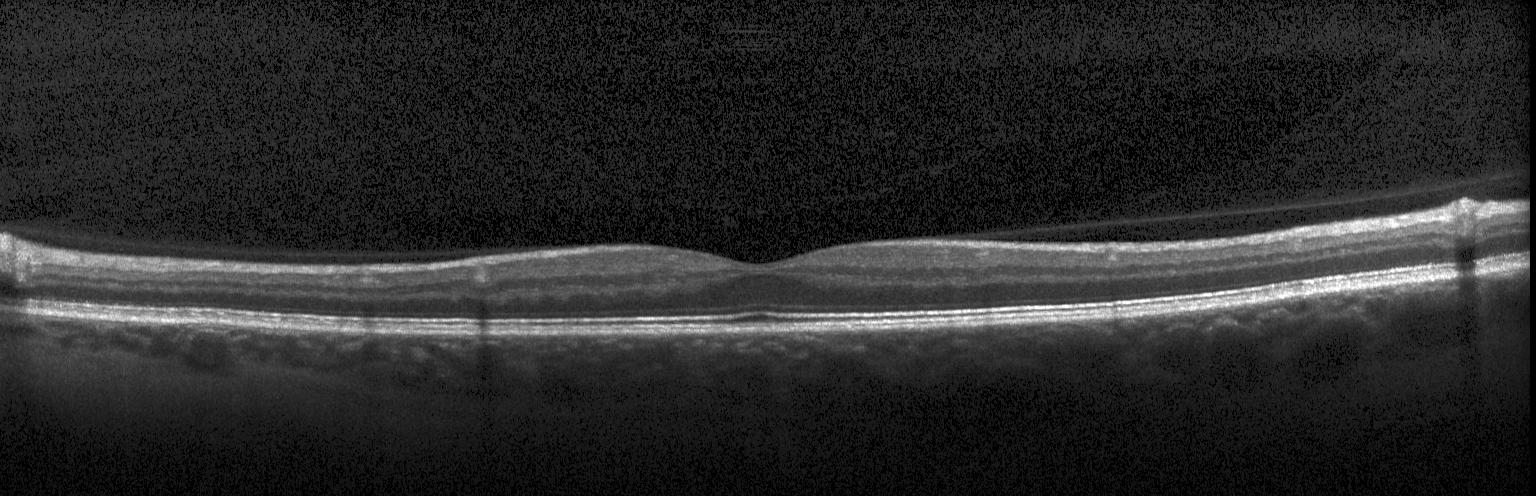 Spectral-domain optical coherence tomography · optical coherence tomography B-scan
Dx: no CNV, DME, or drusen.